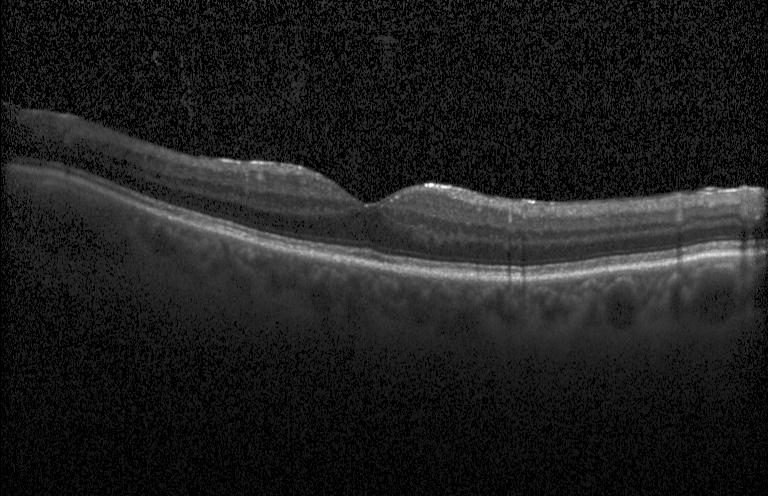
Diagnosis: neither choroidal neovascularization, diabetic macular edema, nor drusen.